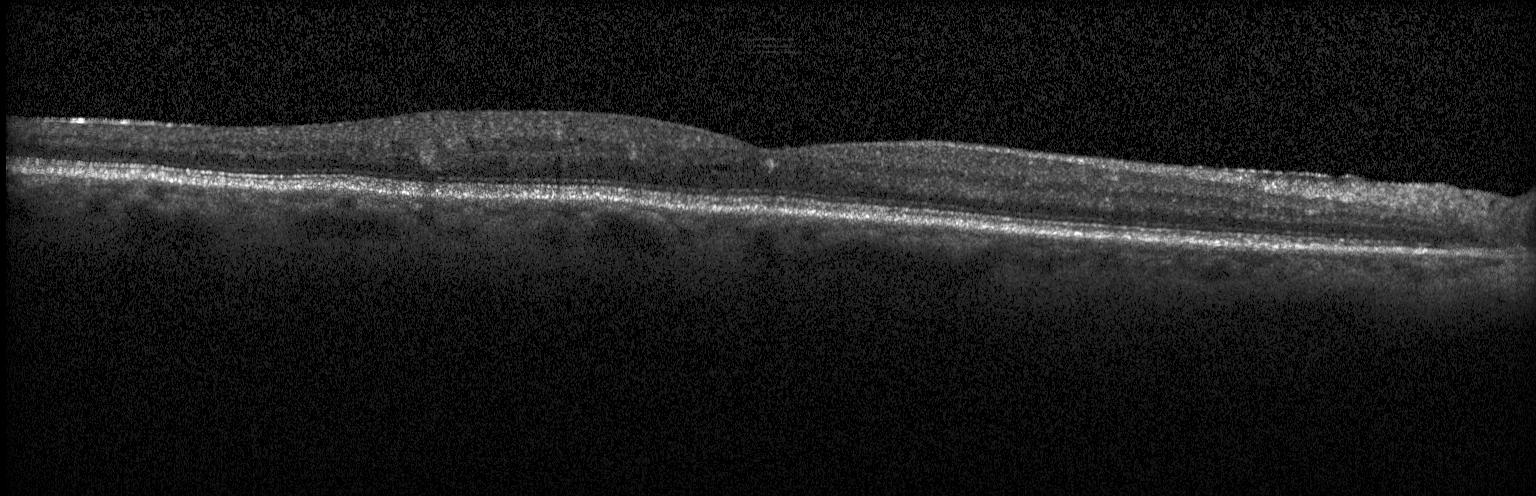 Acquired on a Heidelberg Spectralis, horizontal scan through the fovea, OCT B-scan. Finding: no CNV, DME, or drusen.